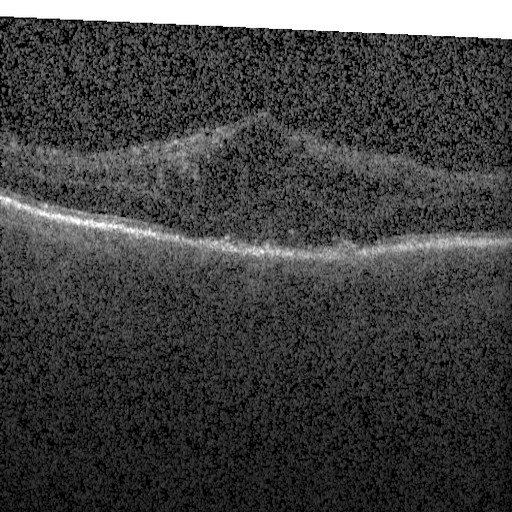
Horizontal scan through the fovea. Acquired on a Heidelberg Spectralis. OCT line scan.
Impression: DME.